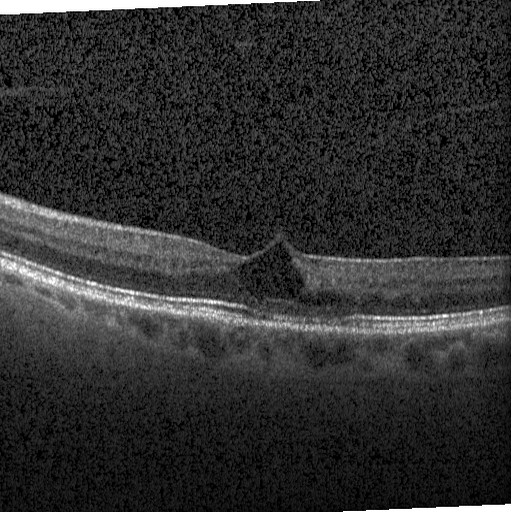 Diagnosis: diabetic macular edema.